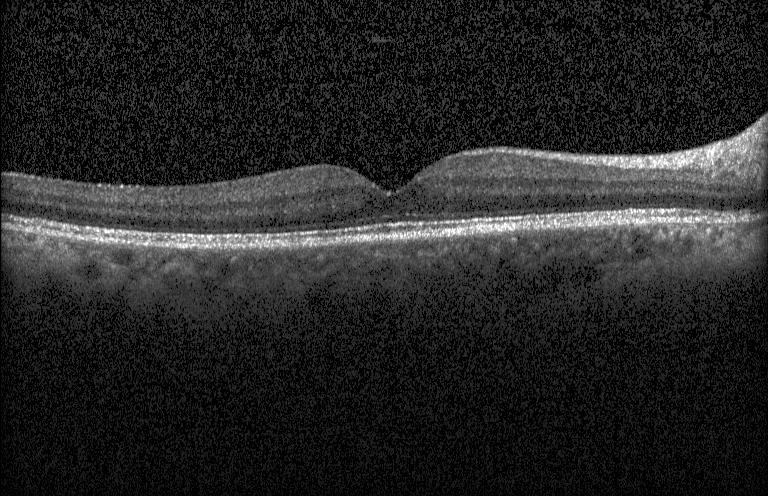 Optical coherence tomography scan — This B-scan demonstrates no choroidal neovascularization, diabetic macular edema, or drusen.